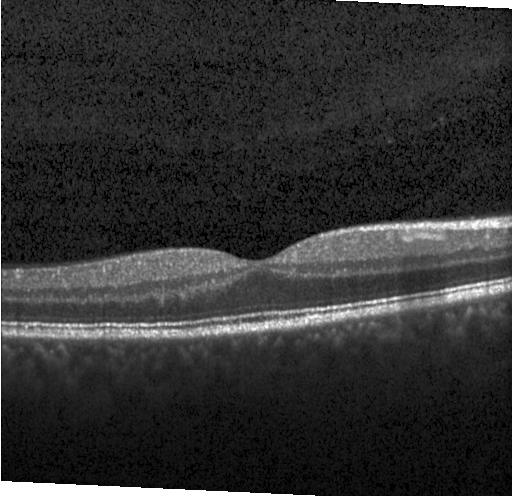 Retinal OCT cross-section showing no choroidal neovascularization, no diabetic macular edema, and no drusen.